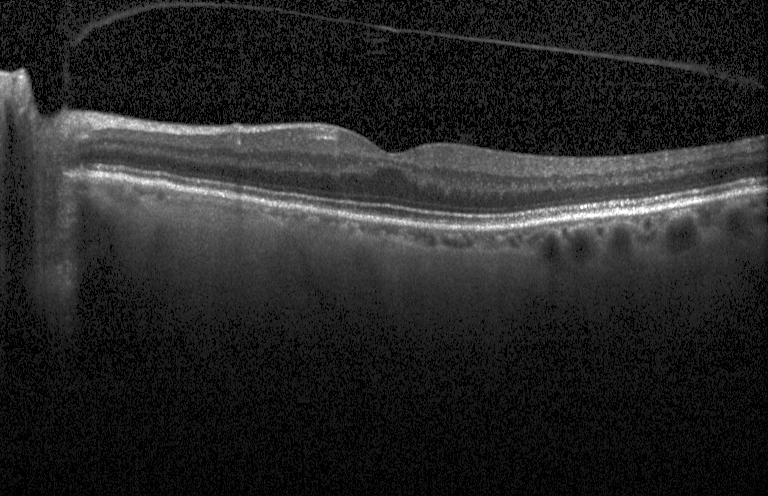
Optical coherence tomography B-scan — Impression: no evidence of choroidal neovascularization, diabetic macular edema, or drusen.